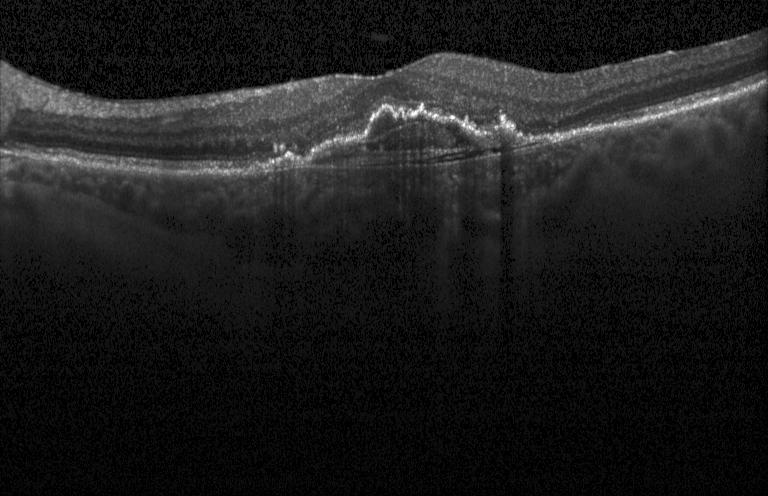

Assessment: a choroidal neovascular membrane.